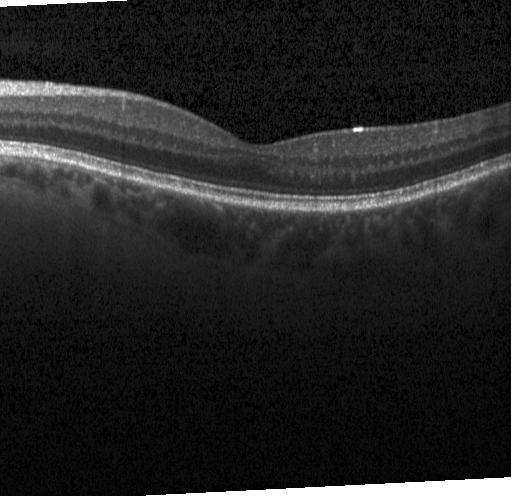
Assessment: no CNV, DME, or drusen.